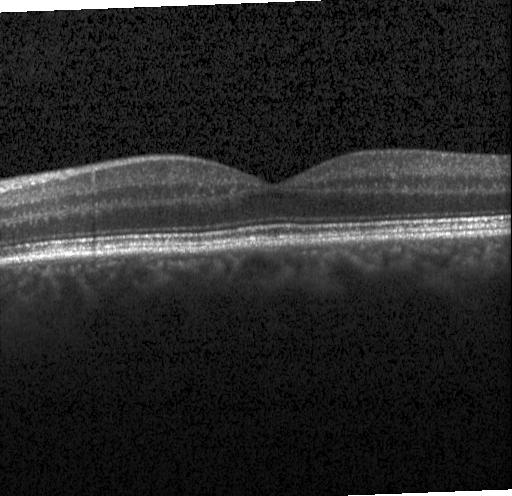

OCT B-scan. Macular OCT: no evidence of choroidal neovascularization, diabetic macular edema, or drusen.